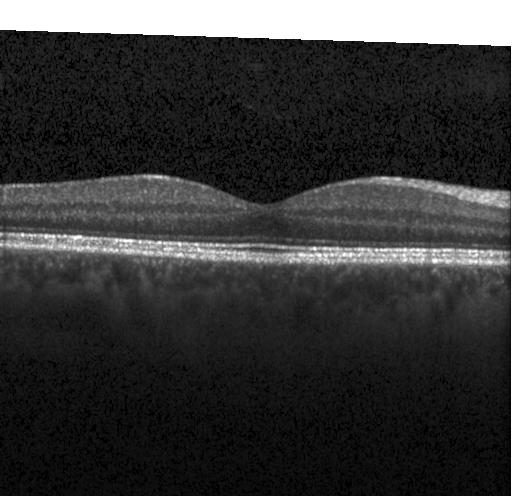

Optical coherence tomography scan
Impression: no evidence of choroidal neovascularization, diabetic macular edema, or drusen.